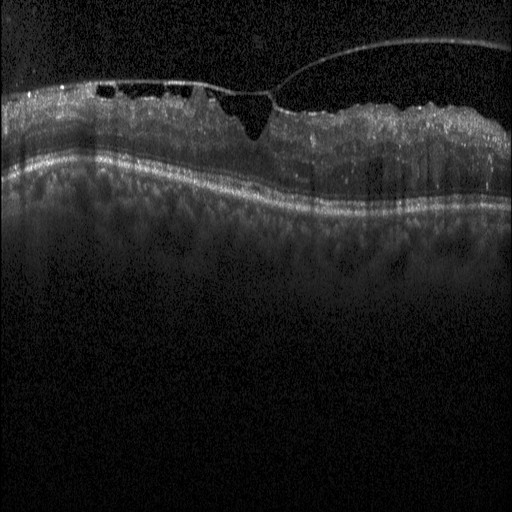
Finding: diabetic macular edema (DME).